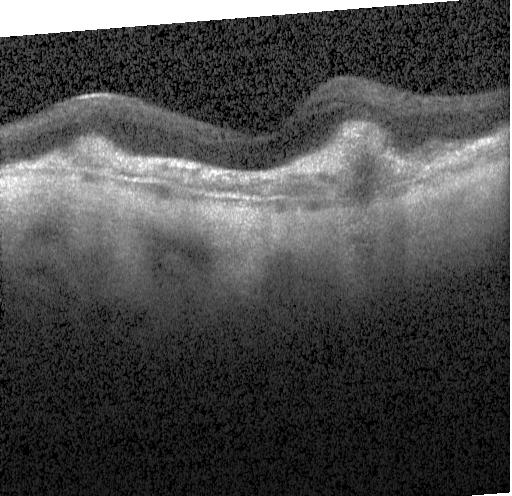
Macular OCT: CNV.